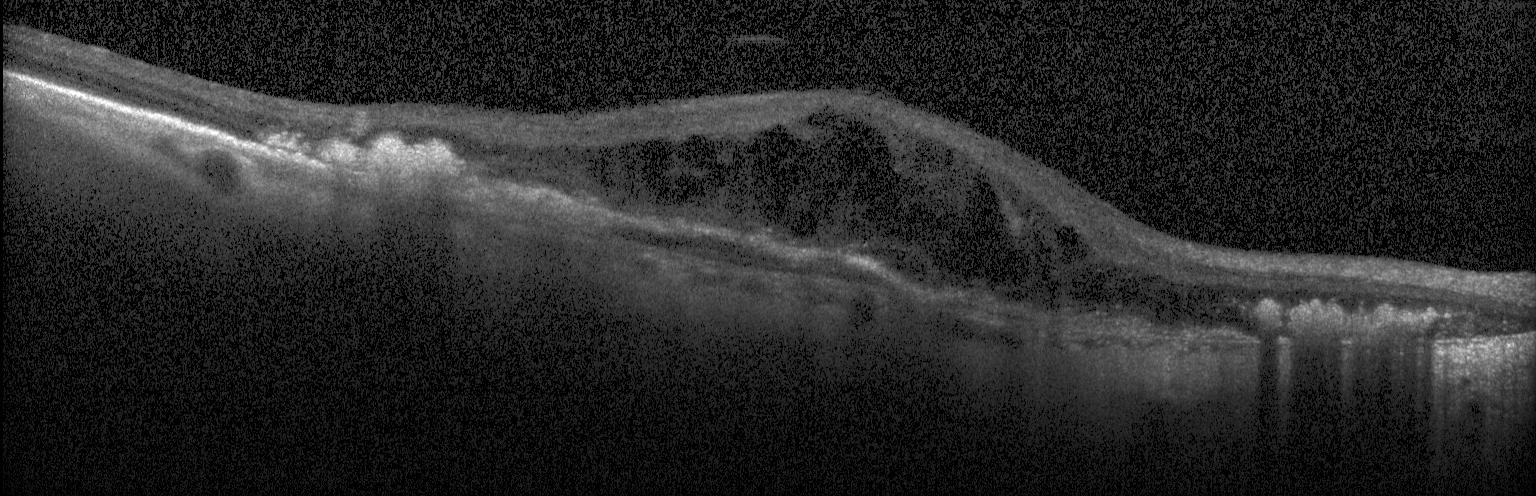
This B-scan demonstrates CNV.